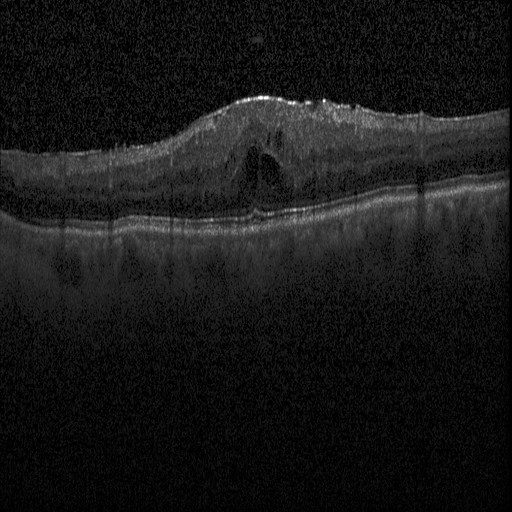

Macular scan · instrument: Heidelberg Spectralis · OCT B-scan — DME.